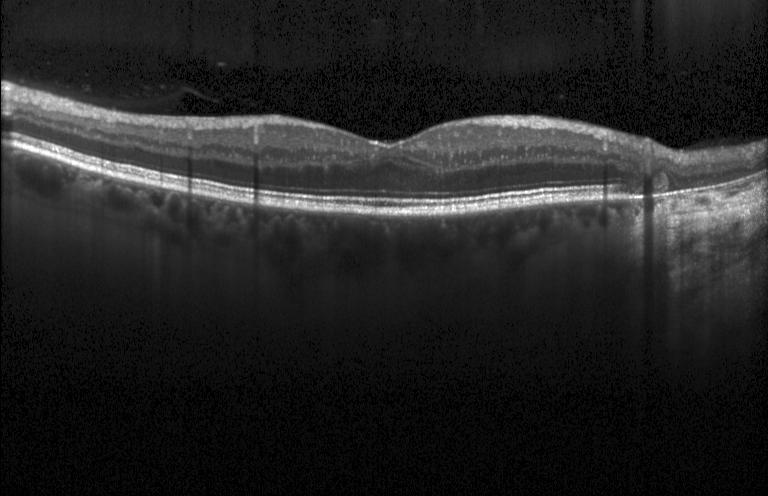
Optical coherence tomography scan — Diagnosis: no evidence of CNV, DME, or drusen.